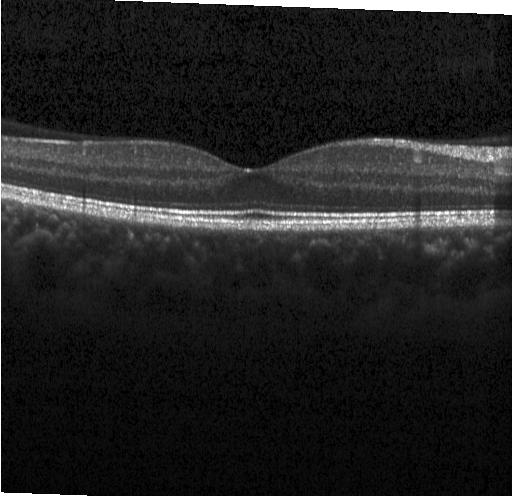

OCT line scan. Diagnosis: neither CNV, DME, nor drusen.